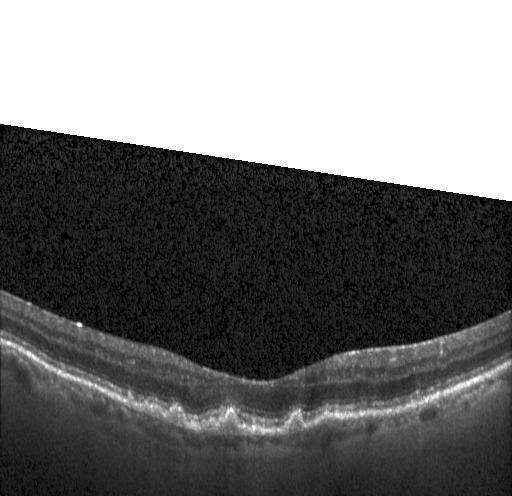 Optical coherence tomography scan. Through the macula. Heidelberg Spectralis OCT system. Spectral-domain optical coherence tomography — Dx: sub-RPE drusenoid deposits.